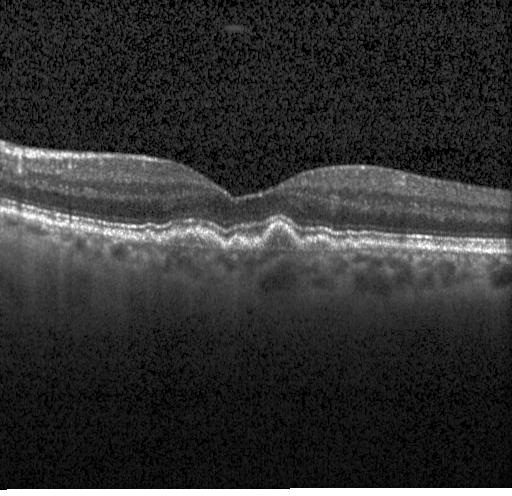
Spectral-domain OCT; horizontal scan through the fovea; Heidelberg Spectralis; retinal OCT B-scan.
Diagnosis: sub-RPE drusenoid deposits.